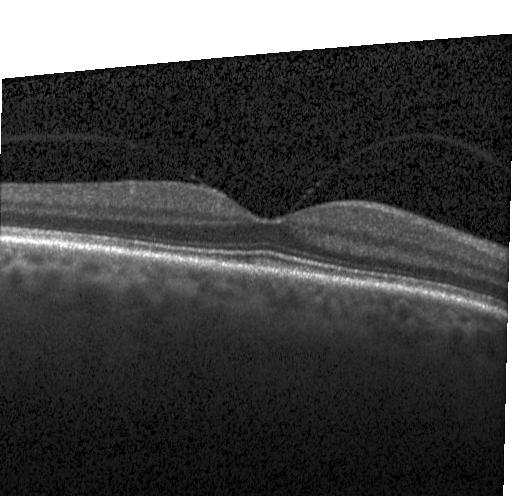

Finding: no evidence of choroidal neovascularization, diabetic macular edema, or drusen.